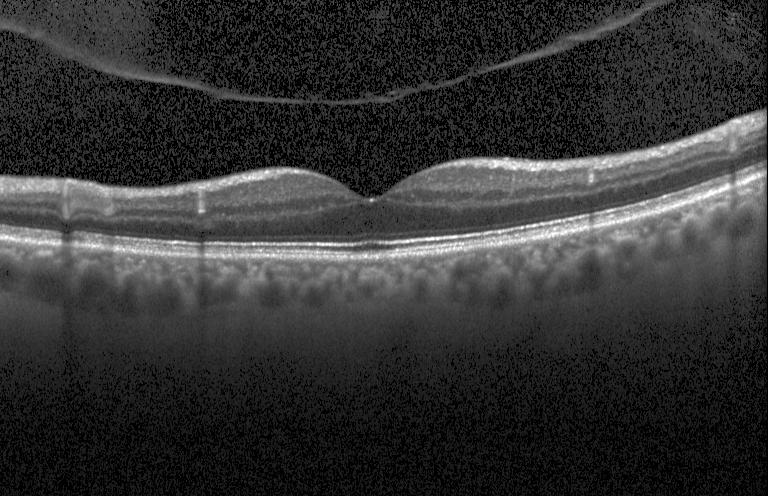
Macular OCT: no CNV, no DME, and no drusen.